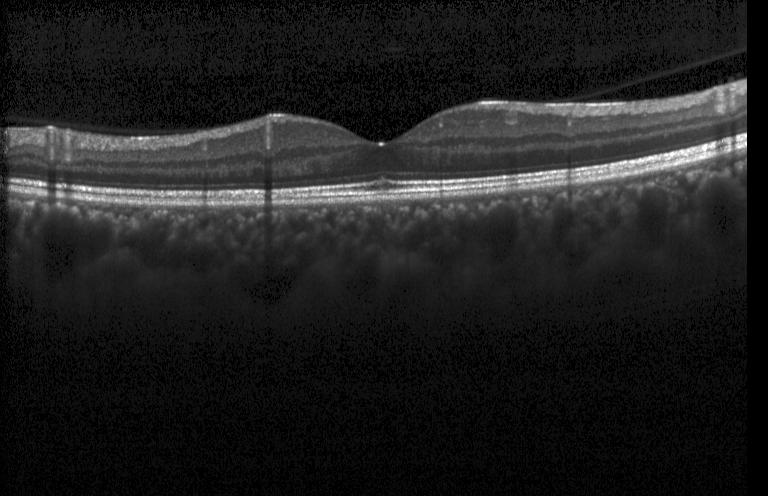 Optical coherence tomography scan, spectral-domain OCT — Impression: no choroidal neovascularization, diabetic macular edema, or drusen.